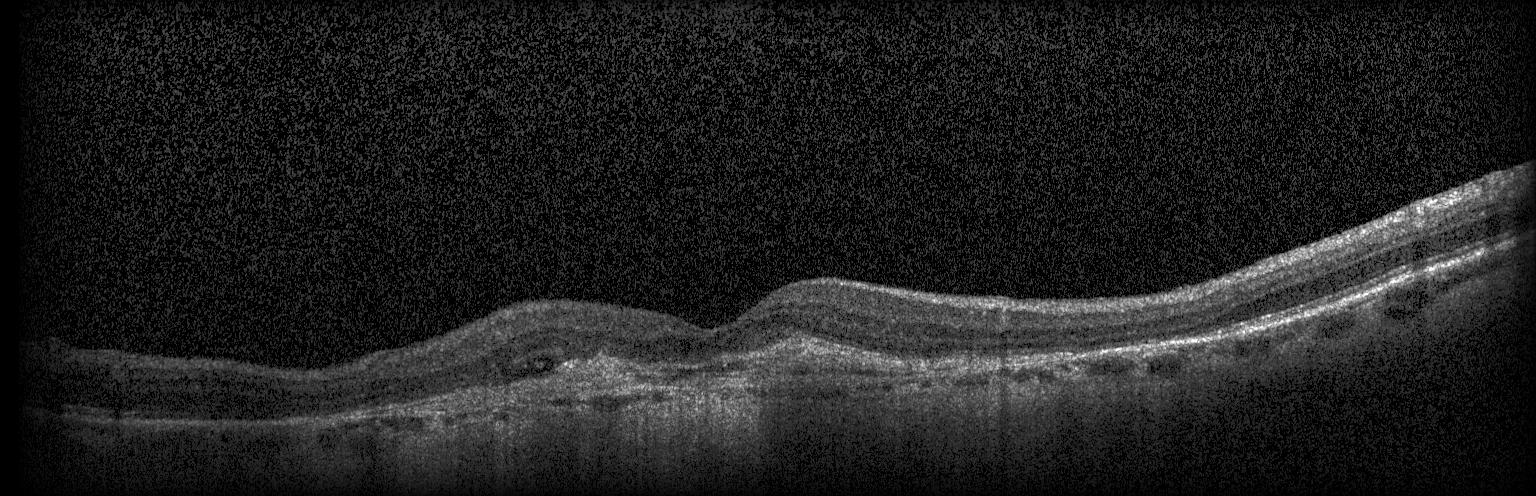

Finding: CNV.